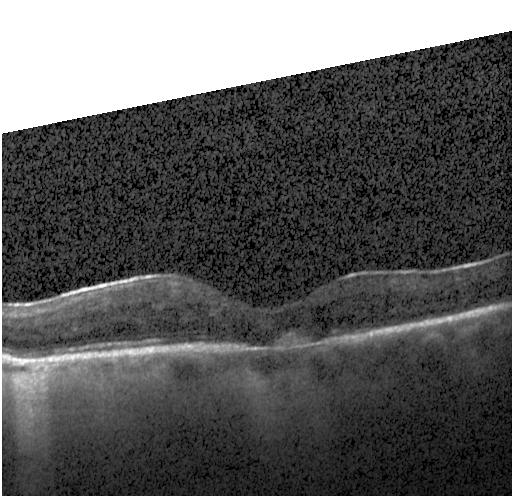

Retinal OCT cross-section. Choroidal neovascularization (CNV).